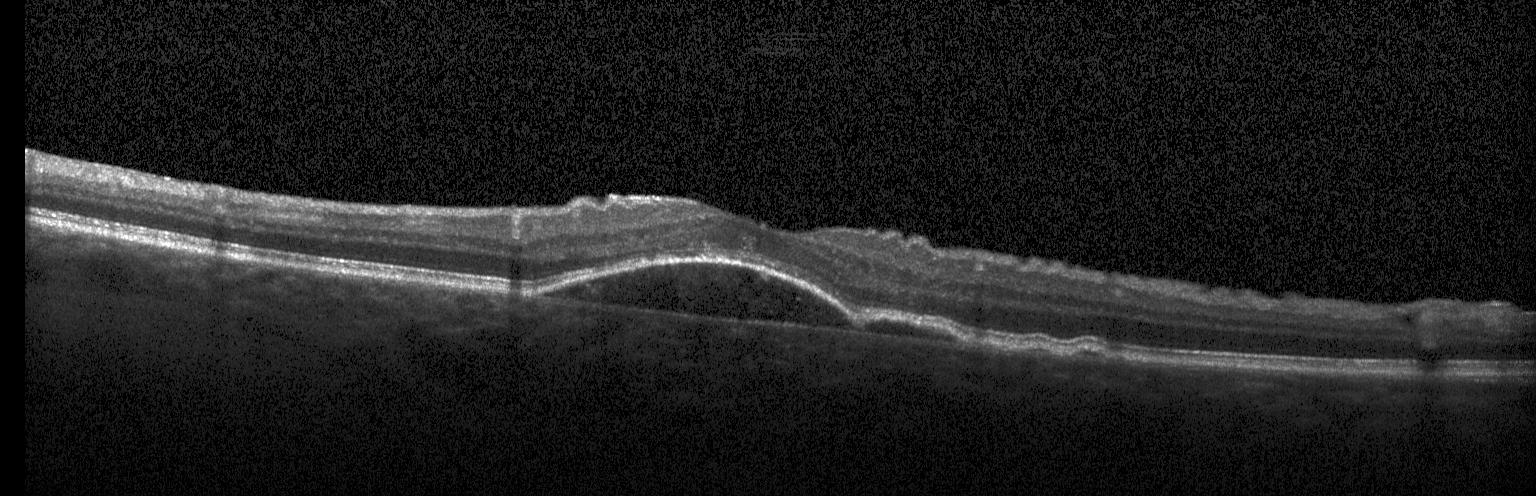 Choroidal neovascularization (CNV).